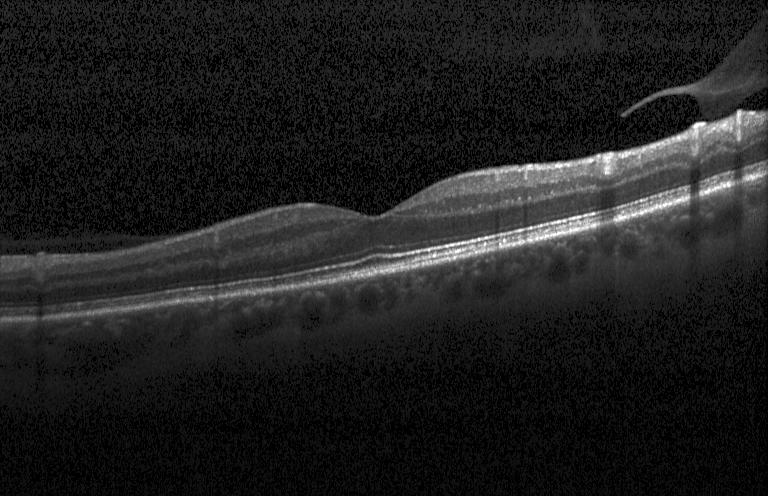
OCT B-scan.
This B-scan demonstrates no choroidal neovascularization, diabetic macular edema, or drusen.